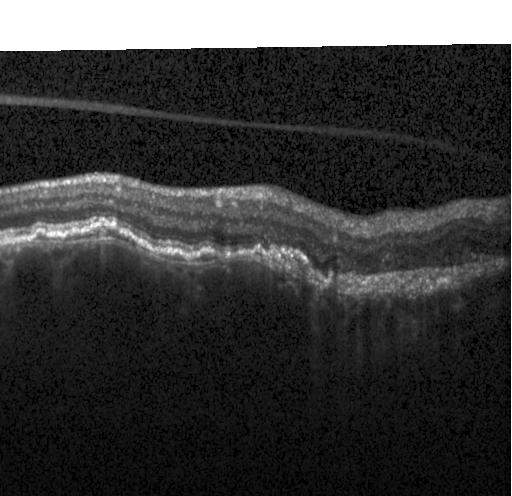

Impression: a choroidal neovascular membrane.